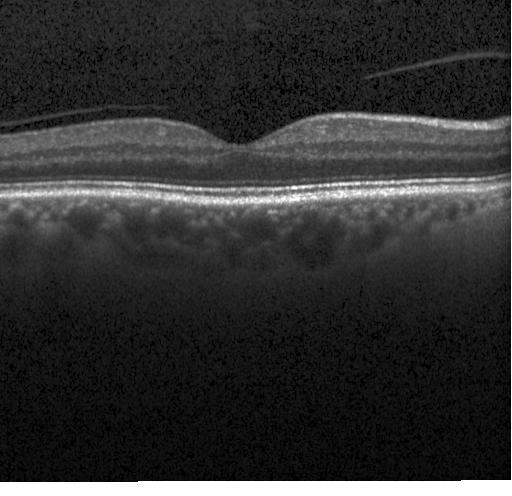 Fovea-centered. Heidelberg Spectralis. OCT line scan — Finding: no evidence of CNV, DME, or drusen.